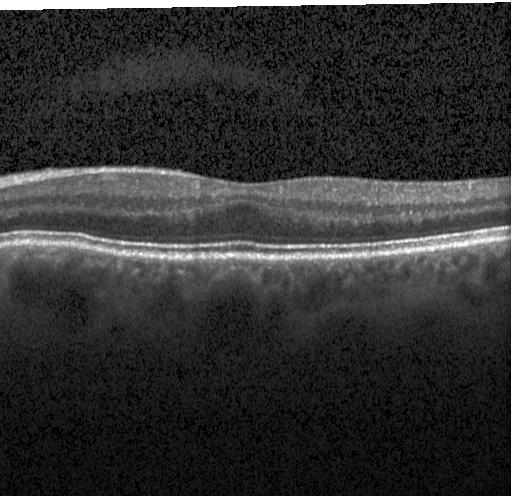 Finding: neither choroidal neovascularization, diabetic macular edema, nor drusen.